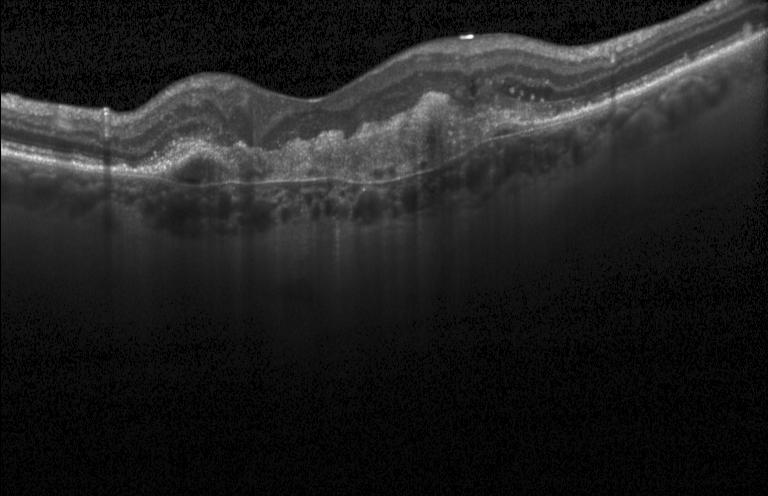
Spectral-domain OCT B-scan: a choroidal neovascular membrane.